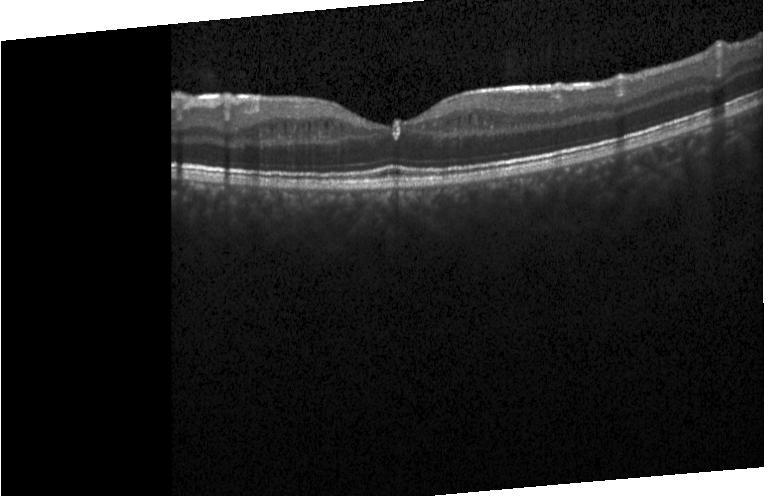

The scan shows diabetic macular edema.